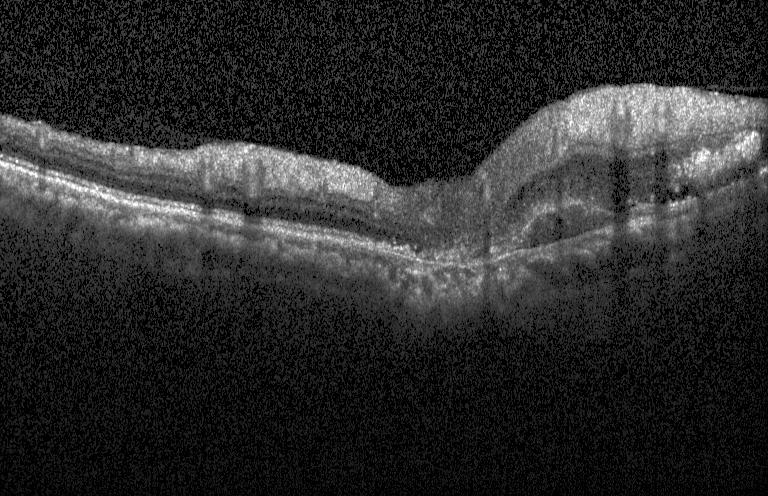

Retinal OCT cross-section.
Choroidal neovascularization.